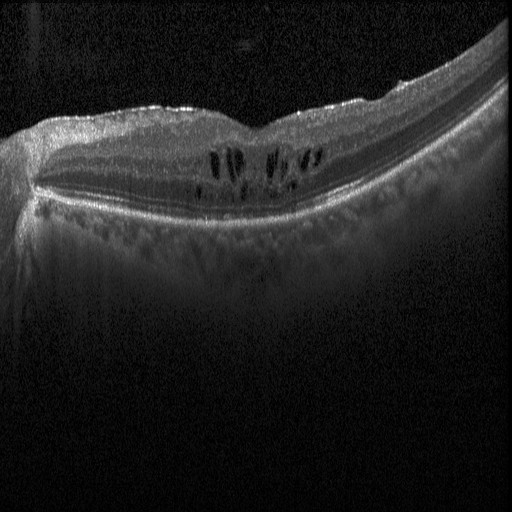 Macular scan. Retinal OCT B-scan. Instrument: Heidelberg Spectralis.
Impression: diabetic macular edema (DME).